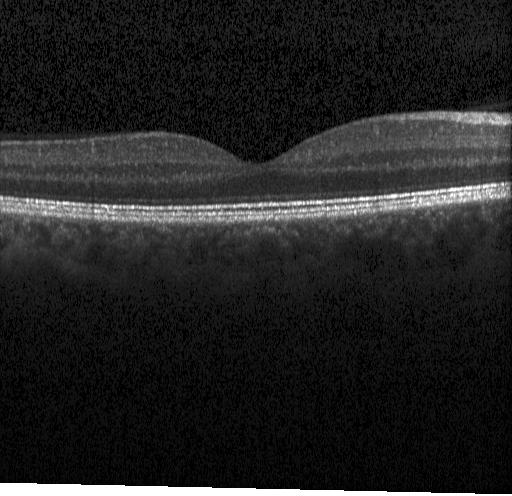
Through the macula. Retinal OCT cross-section
The scan shows no choroidal neovascularization, no diabetic macular edema, and no drusen.